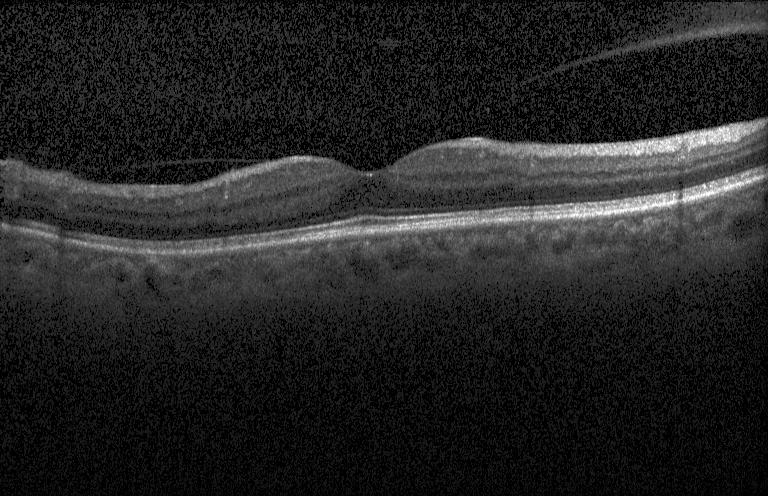

Diagnosis: no choroidal neovascularization, diabetic macular edema, or drusen.